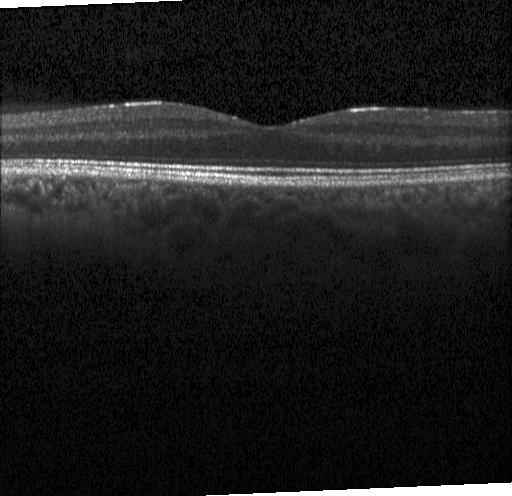

Fovea-centered · Heidelberg Spectralis · optical coherence tomography B-scan. Diagnosis: neither choroidal neovascularization, diabetic macular edema, nor drusen.